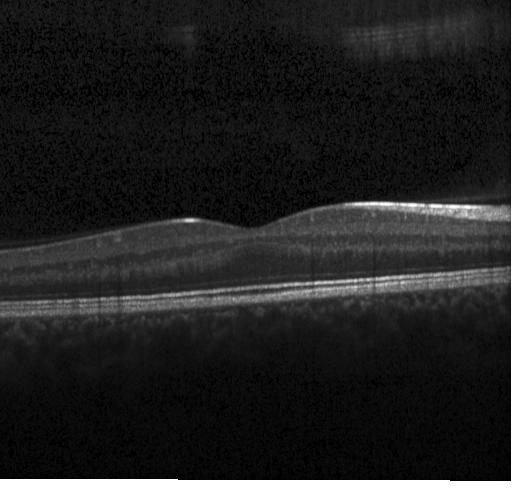 Acquired on a Heidelberg Spectralis, optical coherence tomography scan — Finding: neither choroidal neovascularization, diabetic macular edema, nor drusen.